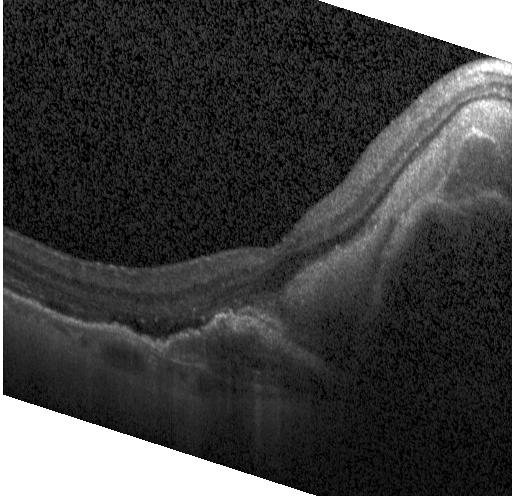 Macular OCT demonstrating a choroidal neovascular membrane.